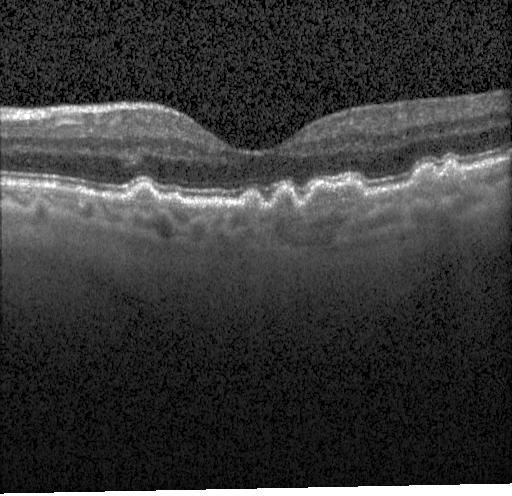

Spectral-domain optical coherence tomography; optical coherence tomography scan; fovea-centered; acquired on a Heidelberg Spectralis — Drusen.